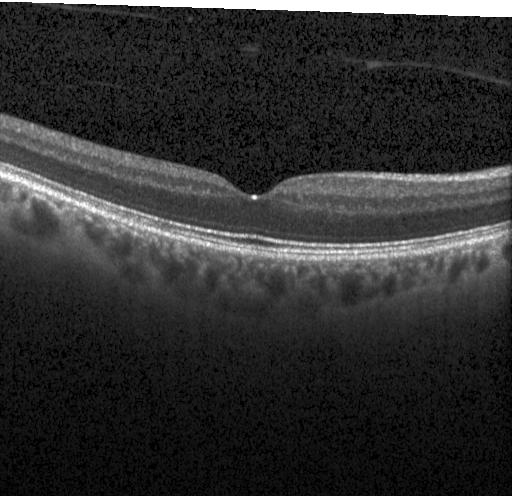
SD-OCT; instrument: Heidelberg Spectralis; retinal OCT B-scan
Finding: no evidence of choroidal neovascularization, diabetic macular edema, or drusen.